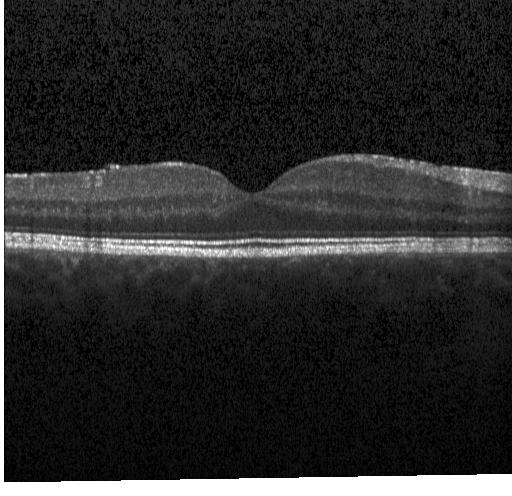

Through the macula. Optical coherence tomography B-scan
Dx: no choroidal neovascularization, diabetic macular edema, or drusen.